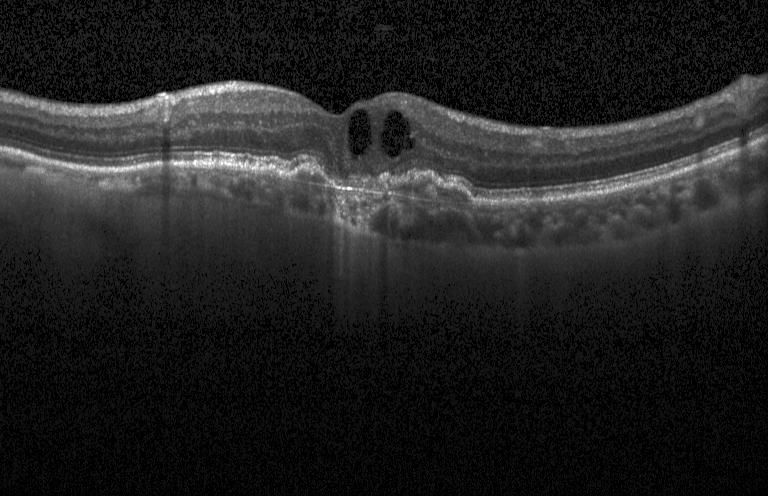

Diagnosis: choroidal neovascularization.